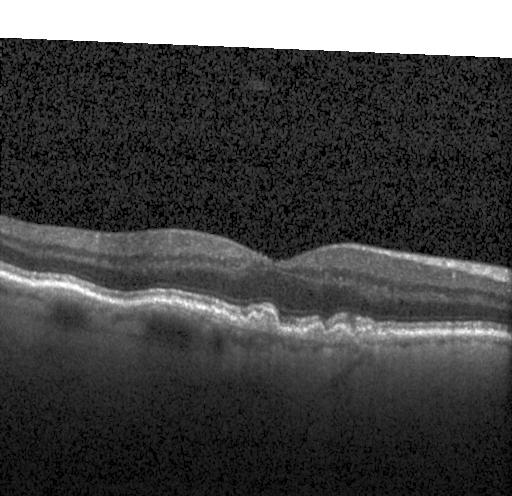
Retinal OCT cross-section — Diagnosis: sub-RPE drusenoid deposits.